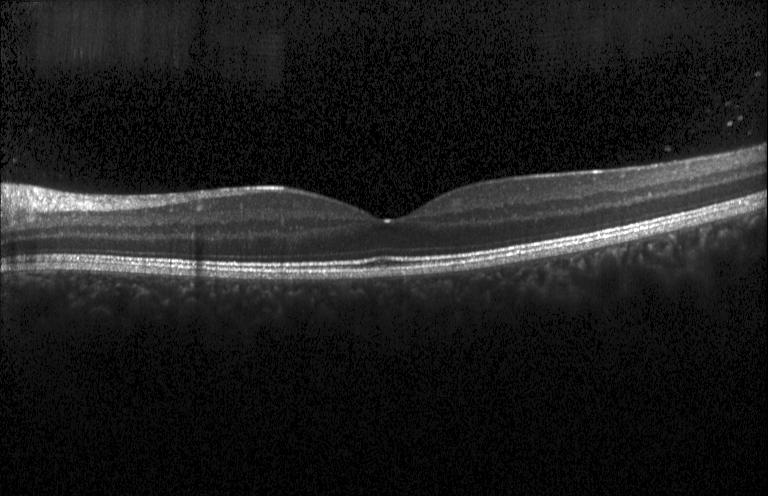
Horizontal scan through the fovea, optical coherence tomography B-scan, Heidelberg Spectralis OCT system.
Diagnosis: no choroidal neovascularization, no diabetic macular edema, and no drusen.